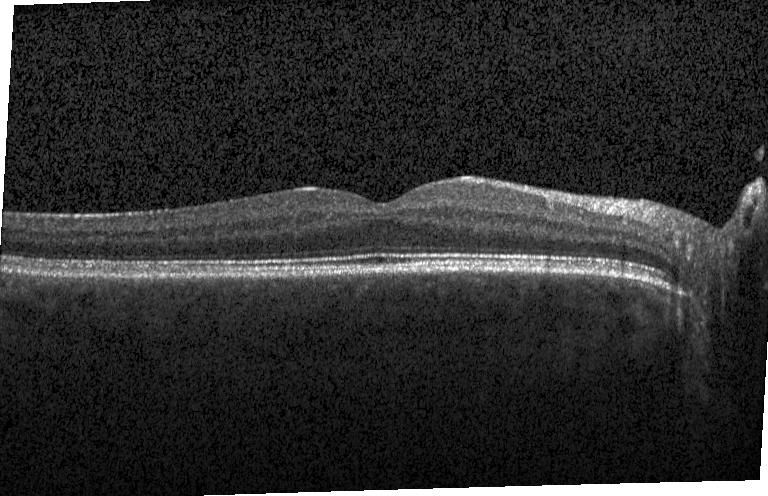

Retinal OCT B-scan
Diagnosis: no choroidal neovascularization, diabetic macular edema, or drusen.